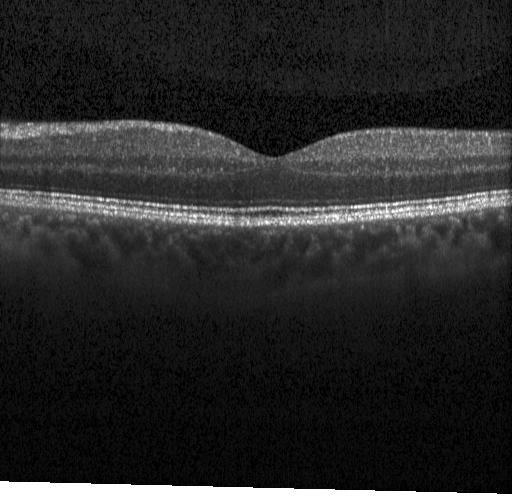
Finding: no evidence of CNV, DME, or drusen.